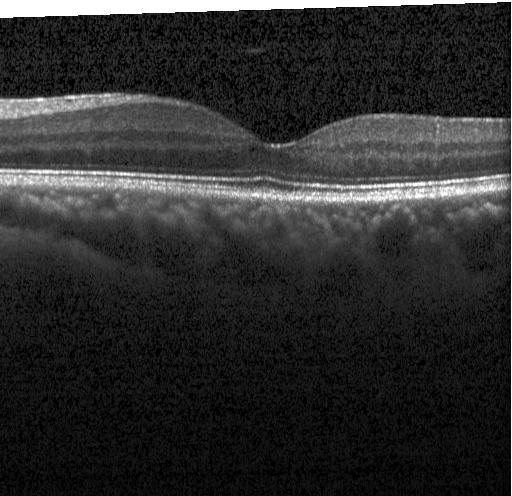

Optical coherence tomography B-scan, centered on the fovea.
Assessment: no choroidal neovascularization, no diabetic macular edema, and no drusen.